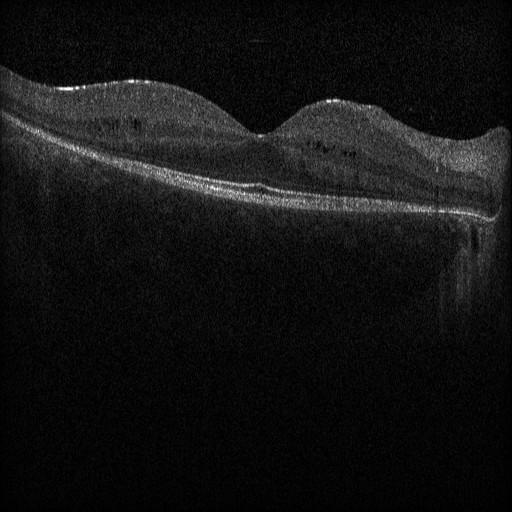

OCT line scan. Heidelberg Spectralis. OCT finding: diabetic macular edema (DME).